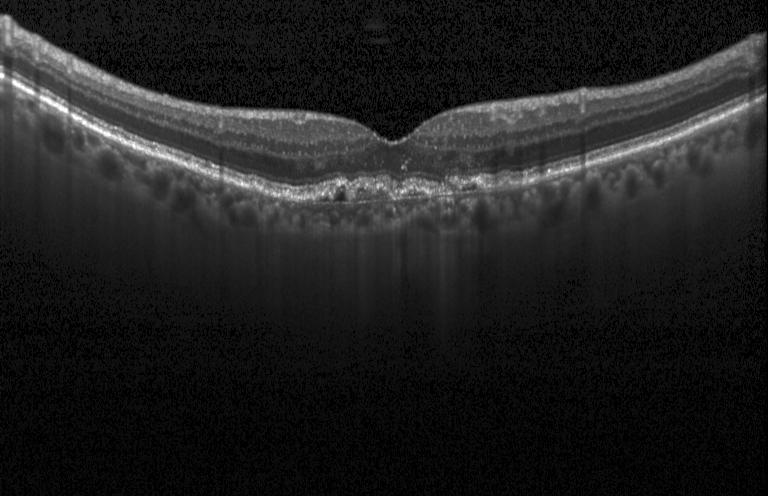

Spectral-domain optical coherence tomography, retinal OCT B-scan — Assessment: CNV.